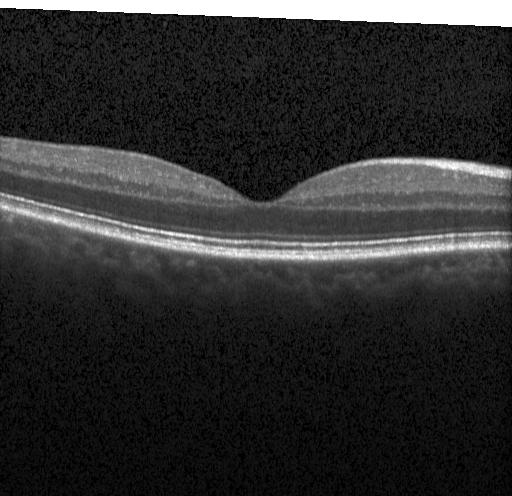
Retinal OCT cross-section; instrument: Heidelberg Spectralis. Diagnosis: no CNV, no DME, and no drusen.